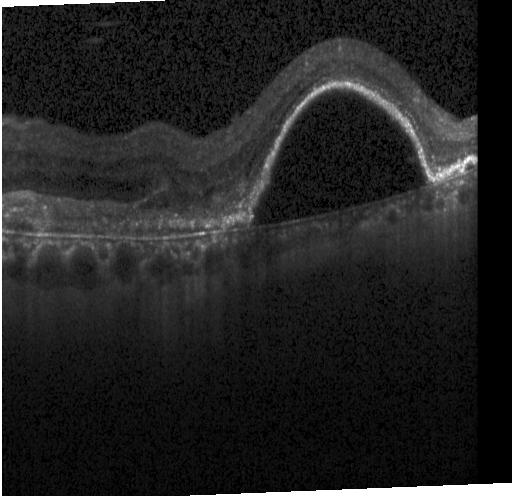
Finding: choroidal neovascularization (CNV).